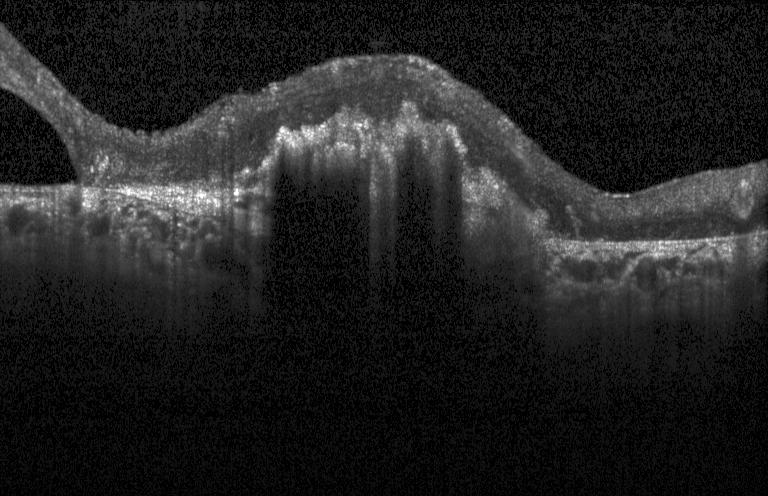

Horizontal scan through the fovea. Retinal OCT cross-section — This B-scan demonstrates choroidal neovascularization.